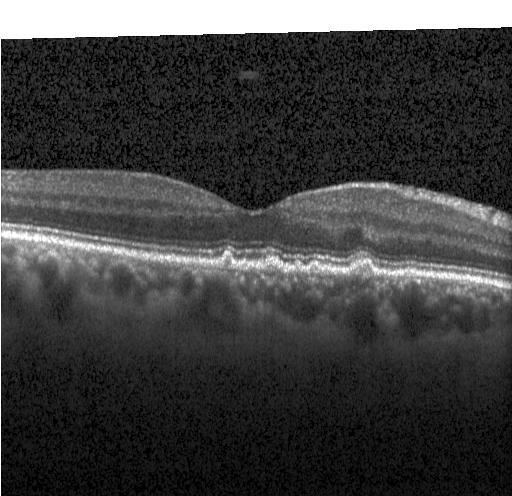 Diagnosis: drusen.